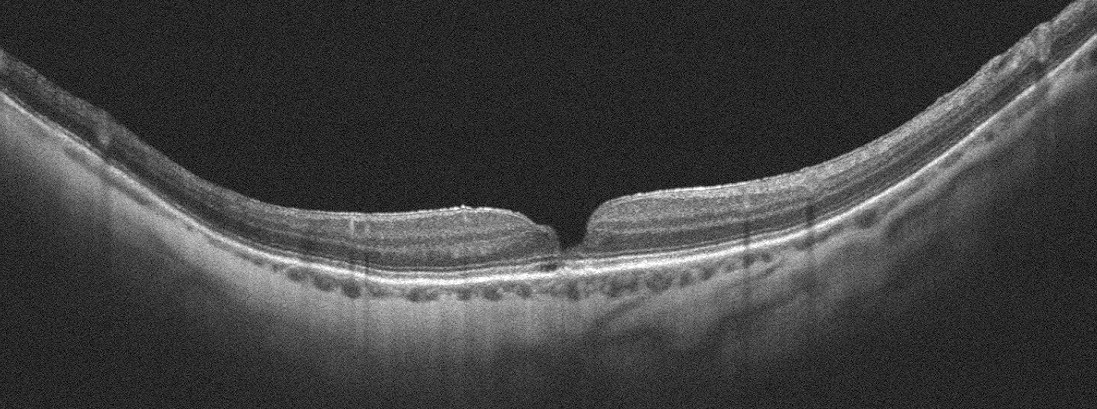
Fovea-centered · acquired on an Optovue Avanti RTVue XR · retinal OCT cross-section.
Epiretinal membrane (ERM).